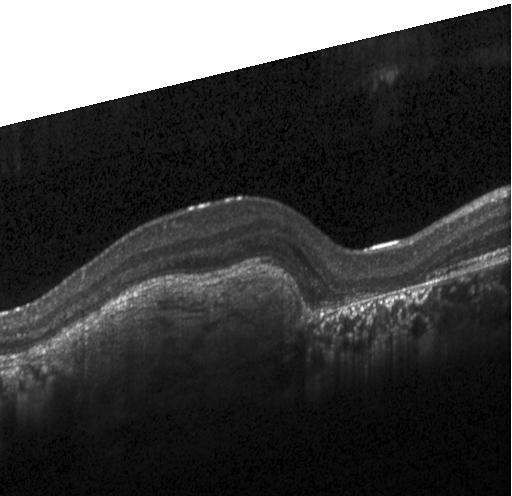 This B-scan demonstrates choroidal neovascularization.